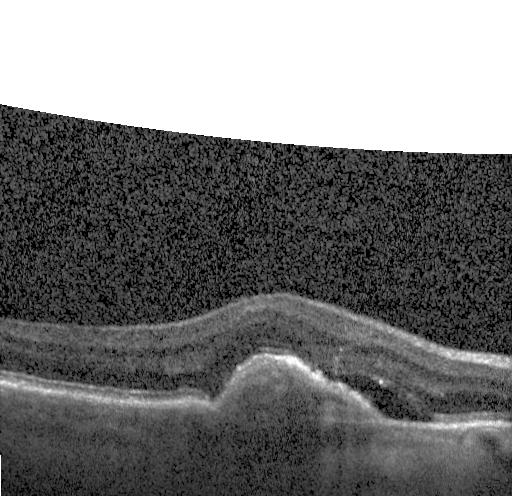
Retinal OCT B-scan · centered on the fovea · spectral-domain OCT
Impression: a choroidal neovascular membrane.